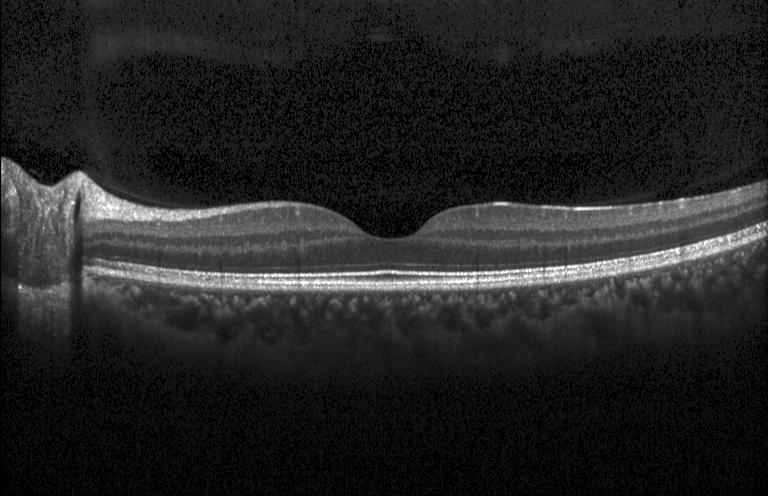 Diagnosis: neither choroidal neovascularization, diabetic macular edema, nor drusen.